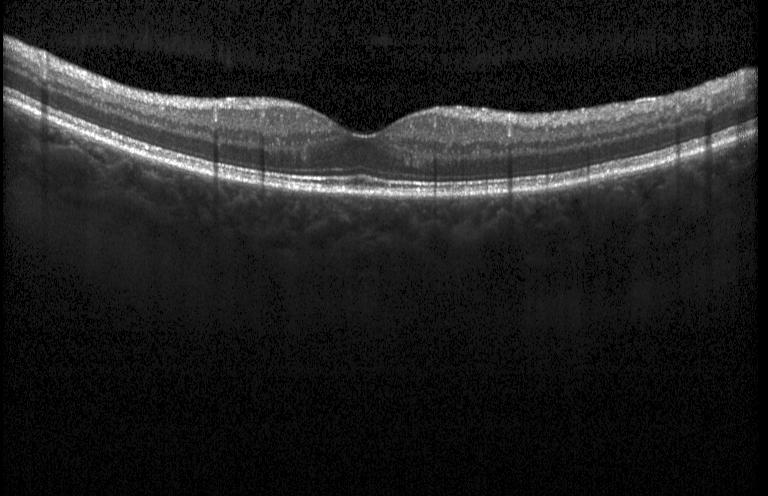

Finding: no evidence of CNV, DME, or drusen.